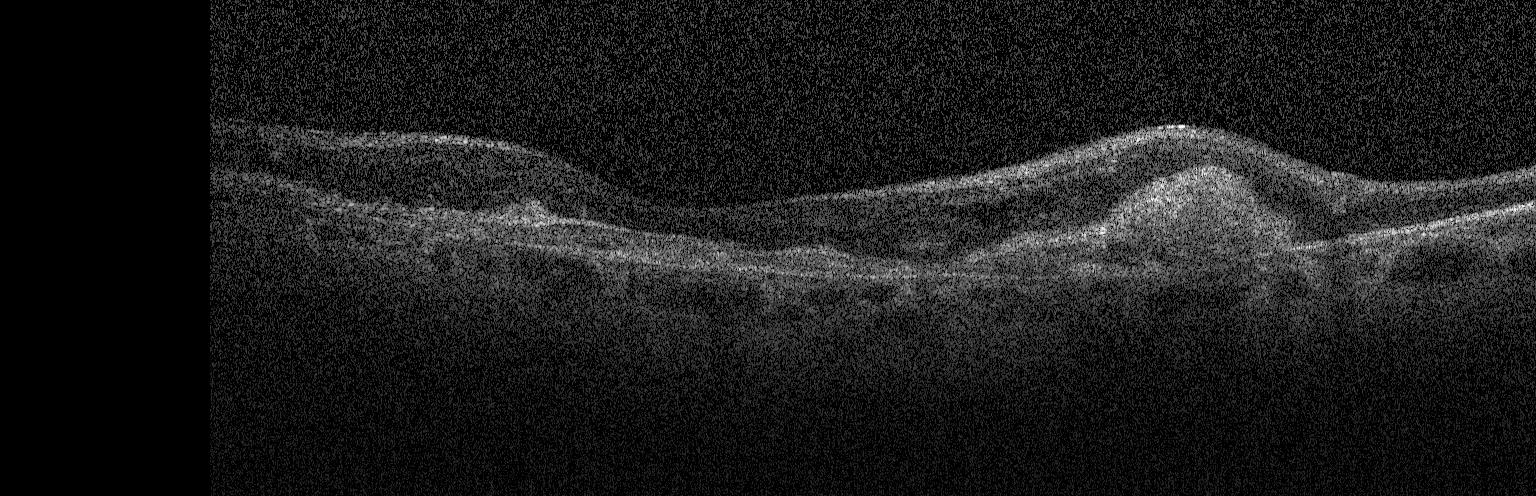
Heidelberg Spectralis, optical coherence tomography scan, spectral-domain OCT.
Impression: a choroidal neovascular membrane.